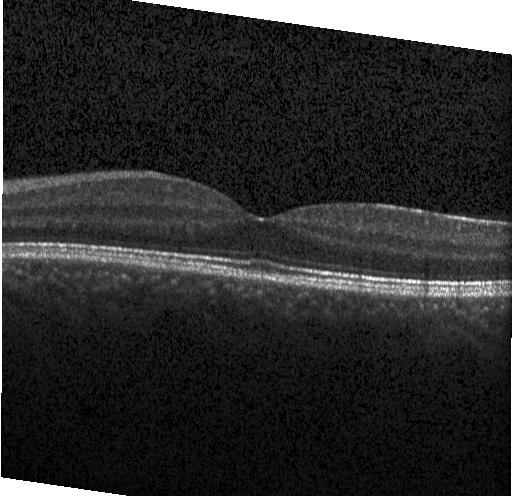

Retinal OCT cross-section — Diagnosis: neither choroidal neovascularization, diabetic macular edema, nor drusen.